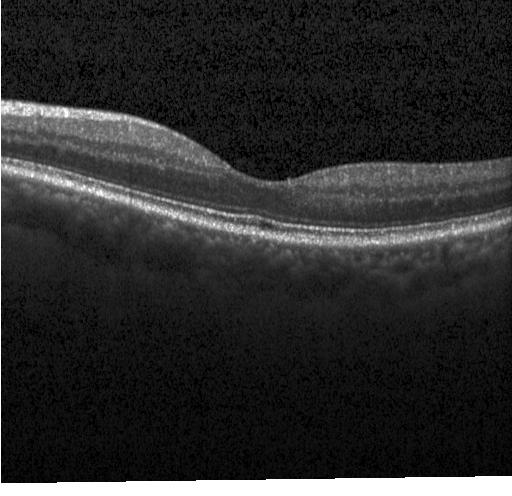
Spectral-domain optical coherence tomography · OCT line scan · horizontal scan through the fovea.
Impression: no choroidal neovascularization, no diabetic macular edema, and no drusen.